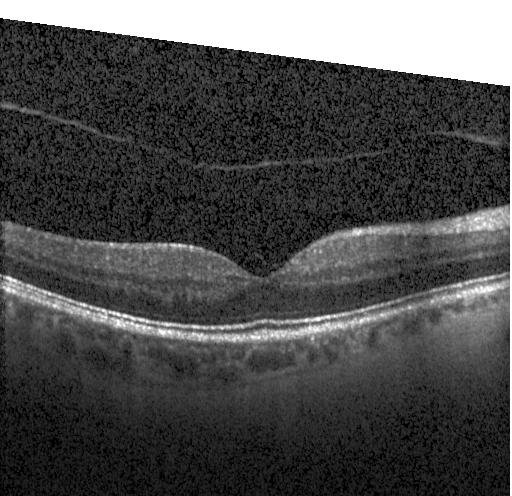 Dx: neither choroidal neovascularization, diabetic macular edema, nor drusen.